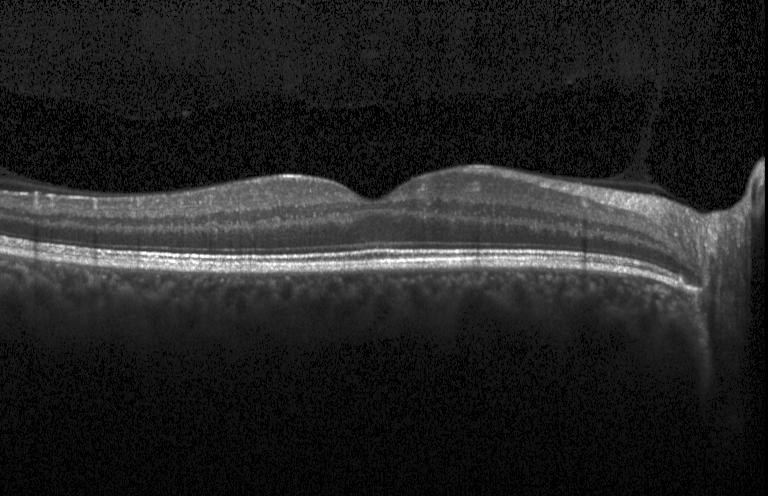
Spectral-domain OCT B-scan: no choroidal neovascularization, diabetic macular edema, or drusen.